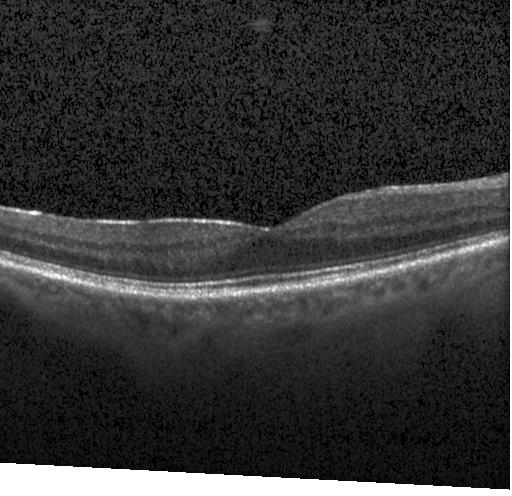 Macular OCT demonstrating no evidence of choroidal neovascularization, diabetic macular edema, or drusen.